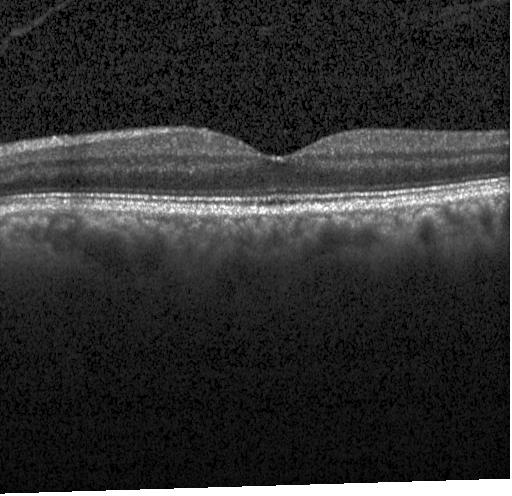 Finding: no choroidal neovascularization, no diabetic macular edema, and no drusen.